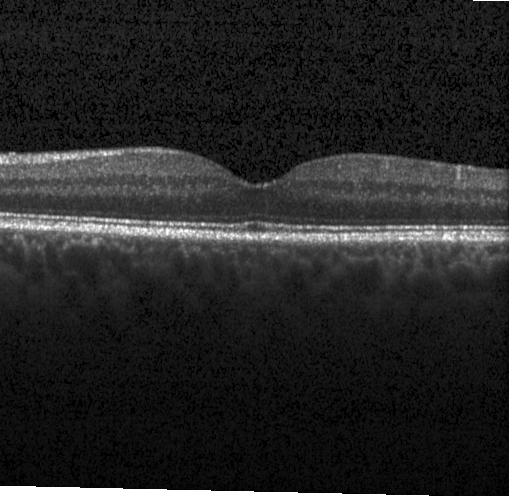
OCT line scan; SD-OCT; instrument: Heidelberg Spectralis; horizontal scan through the fovea
This B-scan demonstrates neither CNV, DME, nor drusen.